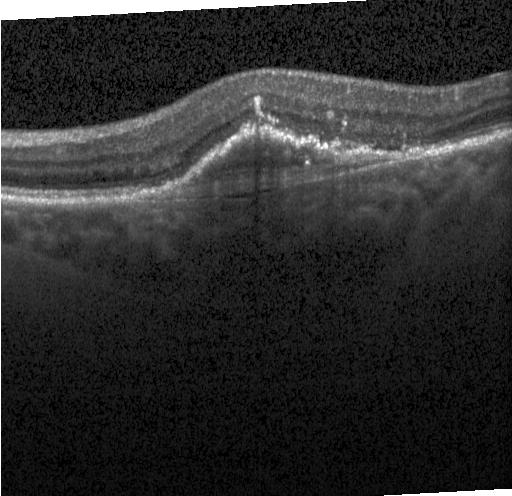

Fovea-centered, OCT line scan, SD-OCT, acquired on a Heidelberg Spectralis.
Macular OCT: choroidal neovascularization.